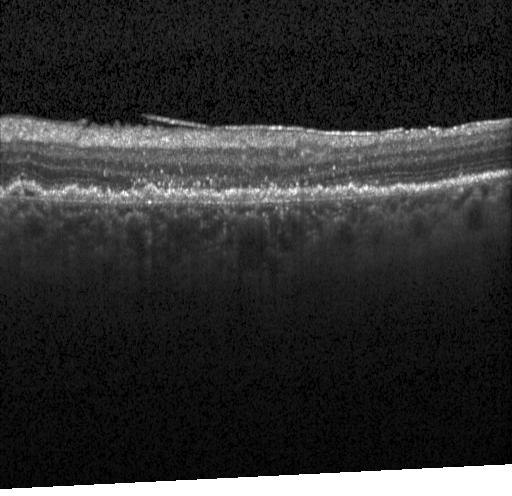

Optical coherence tomography B-scan.
Impression: choroidal neovascularization (CNV).